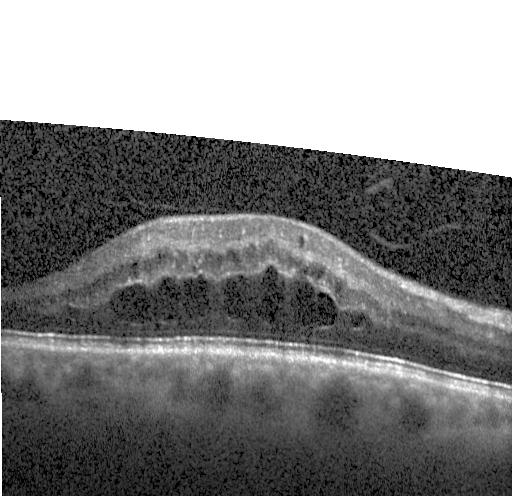 Retinal OCT cross-section showing diabetic macular edema (DME).